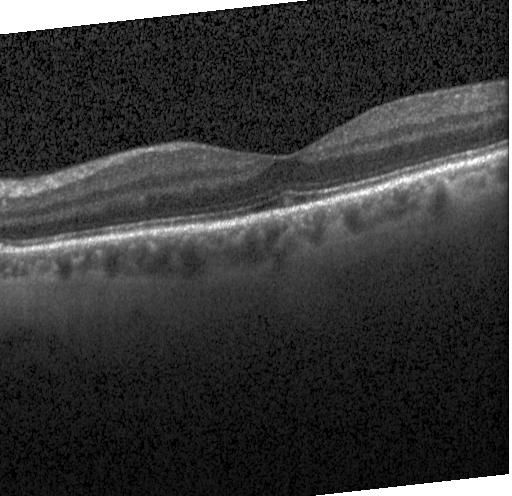 Acquired on a Heidelberg Spectralis. Retinal OCT cross-section. Spectral-domain optical coherence tomography. Fovea-centered.
Diagnosis: neither CNV, DME, nor drusen.